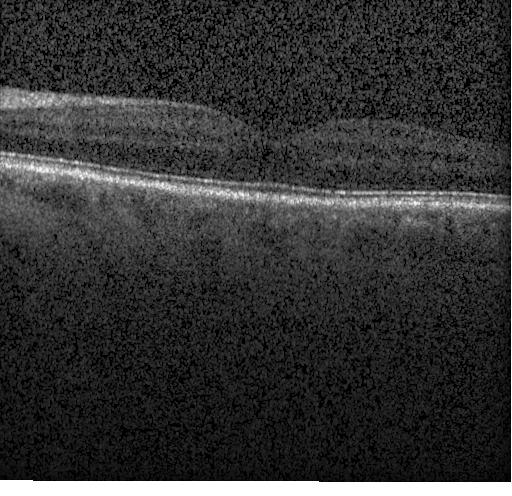
Fovea-centered, optical coherence tomography scan — Diagnosis: no choroidal neovascularization, no diabetic macular edema, and no drusen.